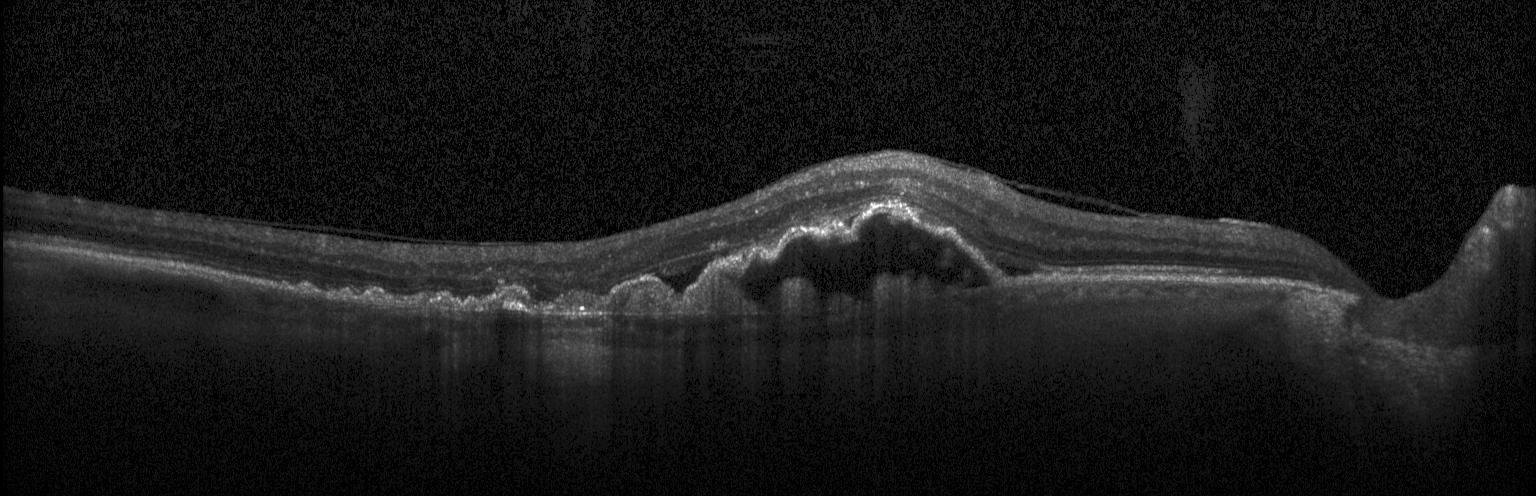 SD-OCT. Optical coherence tomography scan. Macular scan. Heidelberg Spectralis.
This B-scan demonstrates choroidal neovascularization.